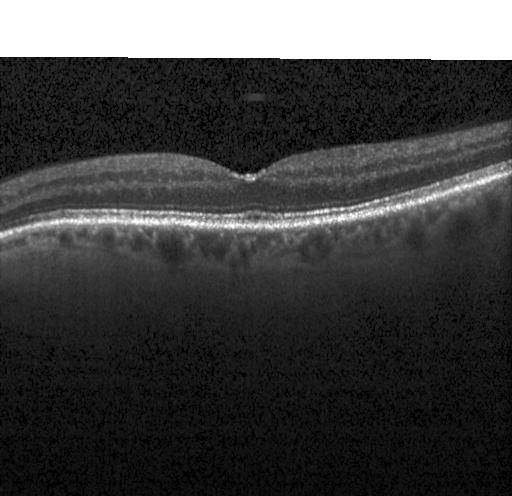
Macular OCT demonstrating no choroidal neovascularization, no diabetic macular edema, and no drusen.